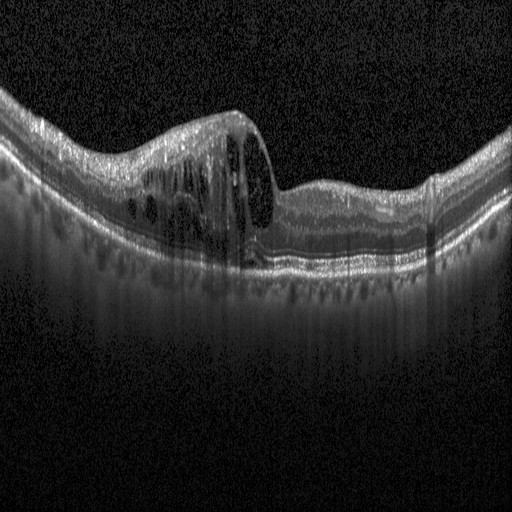
Fovea-centered · Heidelberg Spectralis OCT system · retinal OCT B-scan · SD-OCT.
Finding: diabetic macular edema.